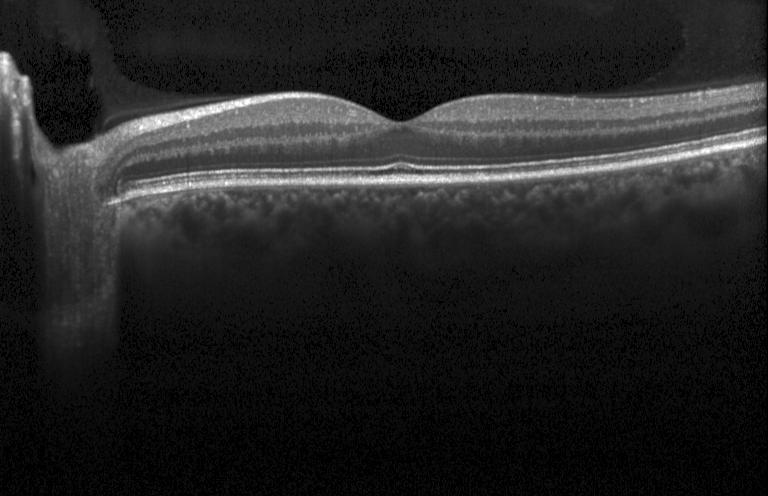 The scan shows no evidence of choroidal neovascularization, diabetic macular edema, or drusen.